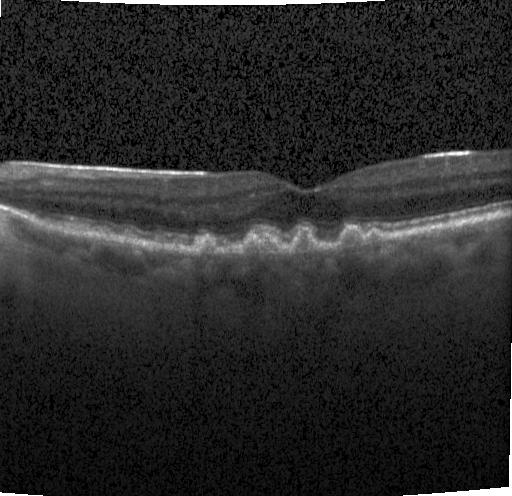
OCT B-scan. Macular OCT: drusen.